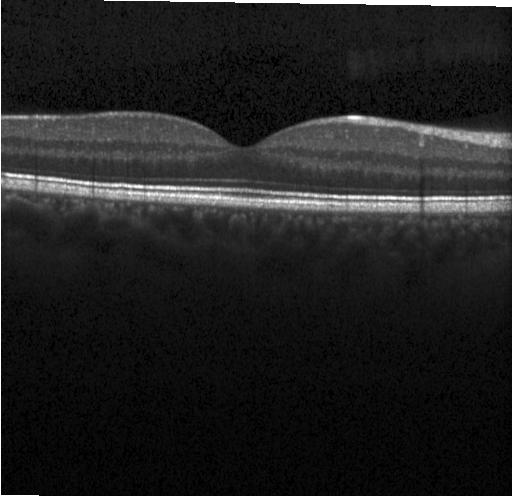
Assessment: no choroidal neovascularization, diabetic macular edema, or drusen.